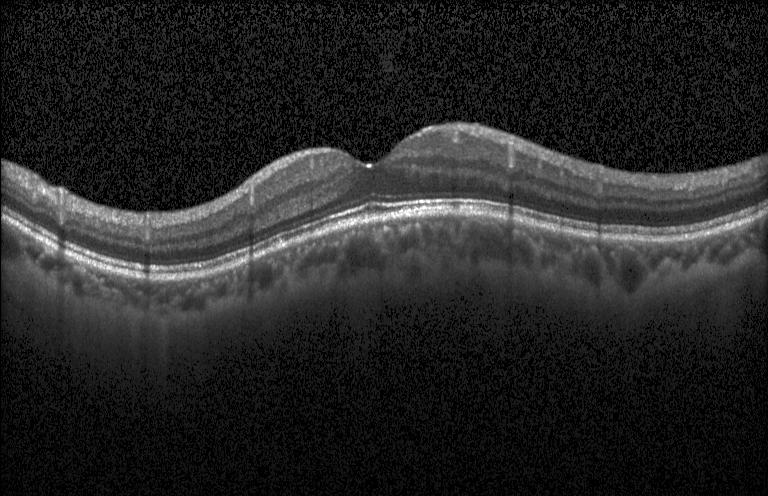

Finding: neither choroidal neovascularization, diabetic macular edema, nor drusen.